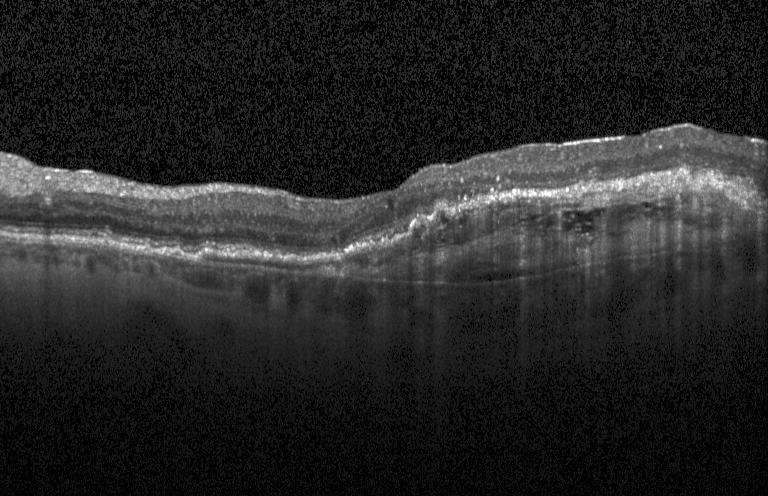
Instrument: Heidelberg Spectralis. SD-OCT. Fovea-centered. OCT B-scan — Macular OCT: choroidal neovascularization.